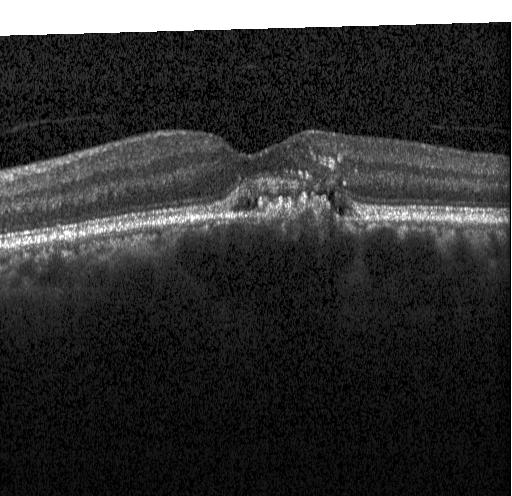

Spectral-domain optical coherence tomography; OCT line scan; instrument: Heidelberg Spectralis; centered on the fovea
OCT finding: choroidal neovascularization (CNV).